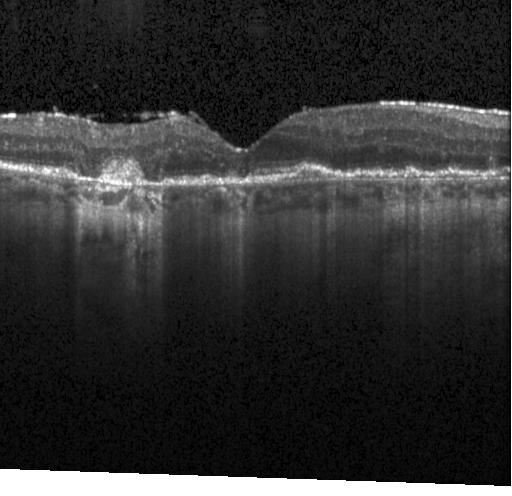
Fovea-centered; retinal OCT cross-section.
Diagnosis: a choroidal neovascular membrane.